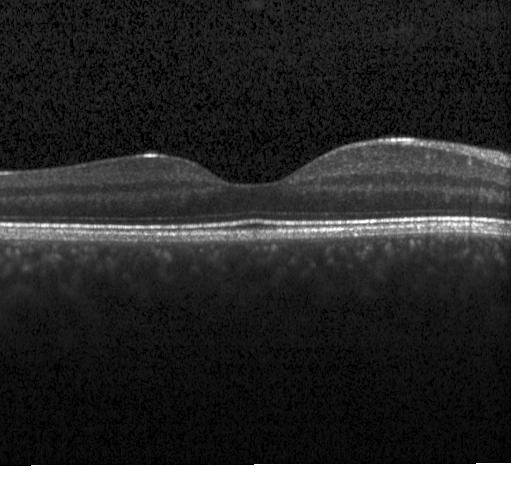

OCT B-scan · Heidelberg Spectralis OCT system
Finding: neither choroidal neovascularization, diabetic macular edema, nor drusen.